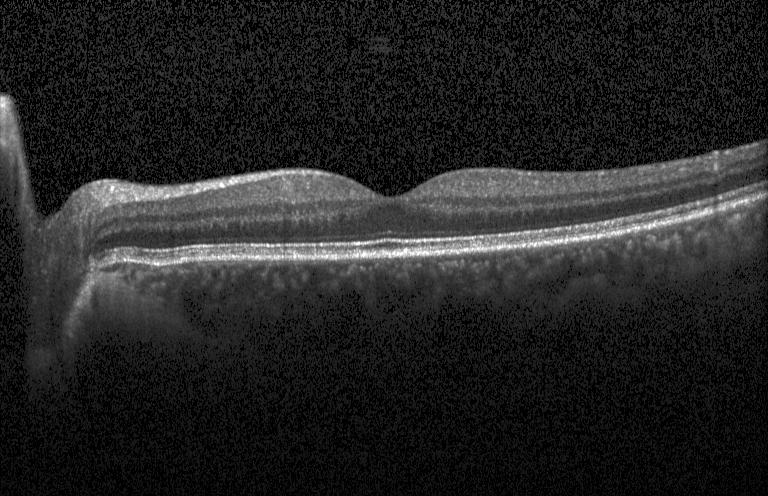
Dx: neither choroidal neovascularization, diabetic macular edema, nor drusen.